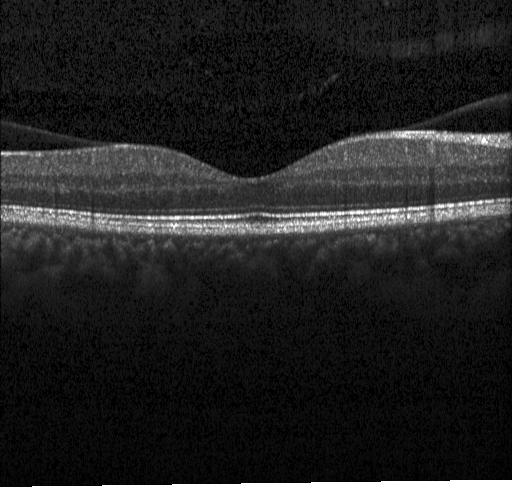

Heidelberg Spectralis OCT system. Spectral-domain OCT. Centered on the fovea. Retinal OCT cross-section
OCT finding: no choroidal neovascularization, no diabetic macular edema, and no drusen.